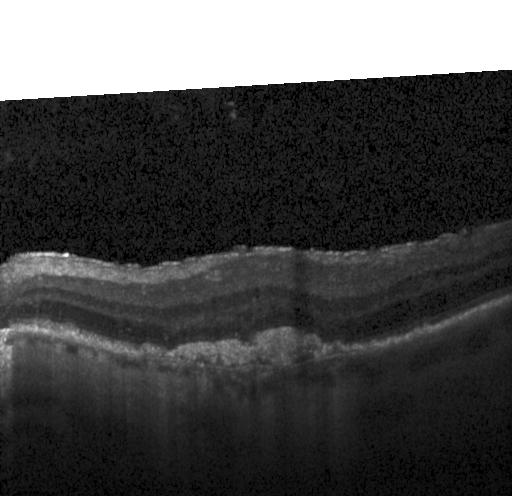

OCT finding: a choroidal neovascular membrane.